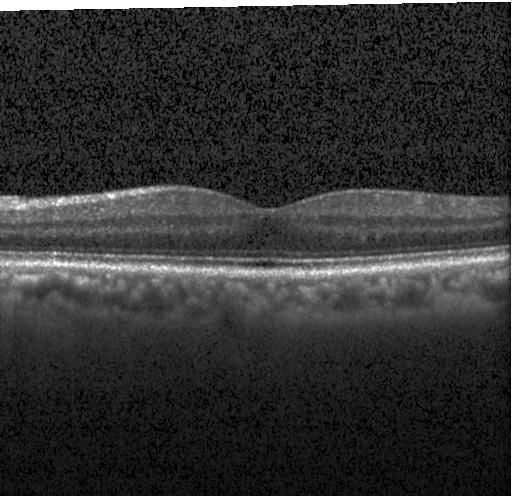
OCT line scan.
Macular OCT: no CNV, DME, or drusen.